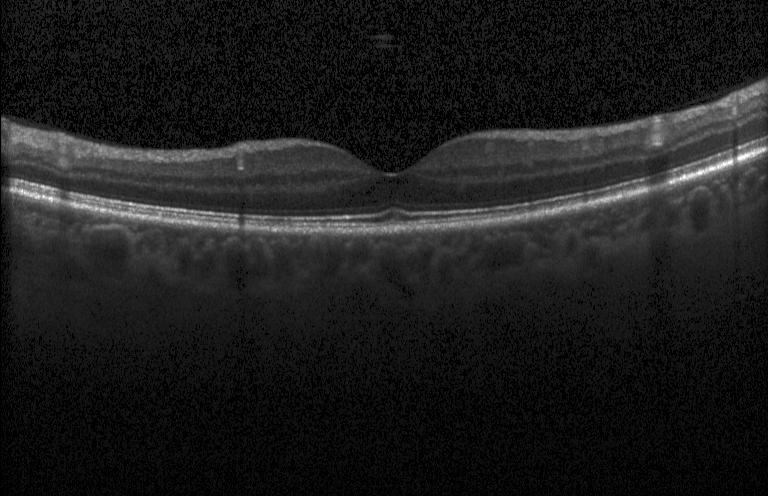
Diagnosis: no choroidal neovascularization, diabetic macular edema, or drusen.